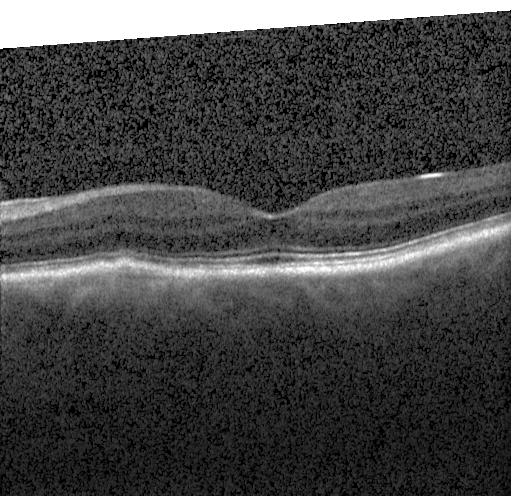 Optical coherence tomography scan — Drusen.